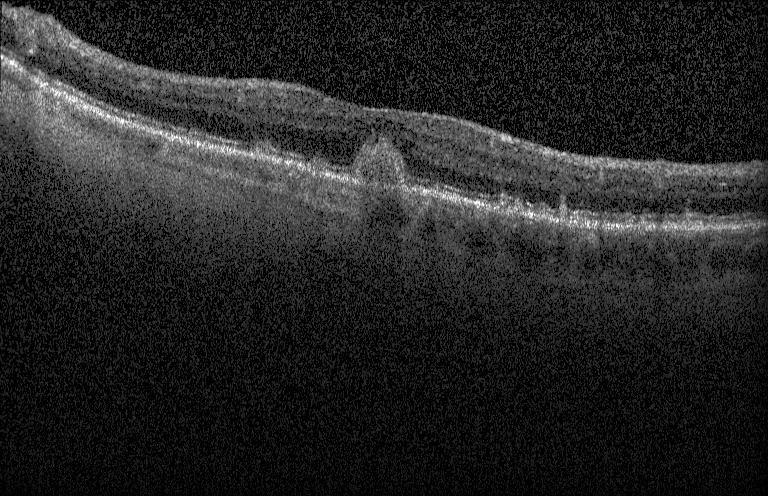 OCT line scan. OCT finding: choroidal neovascularization.